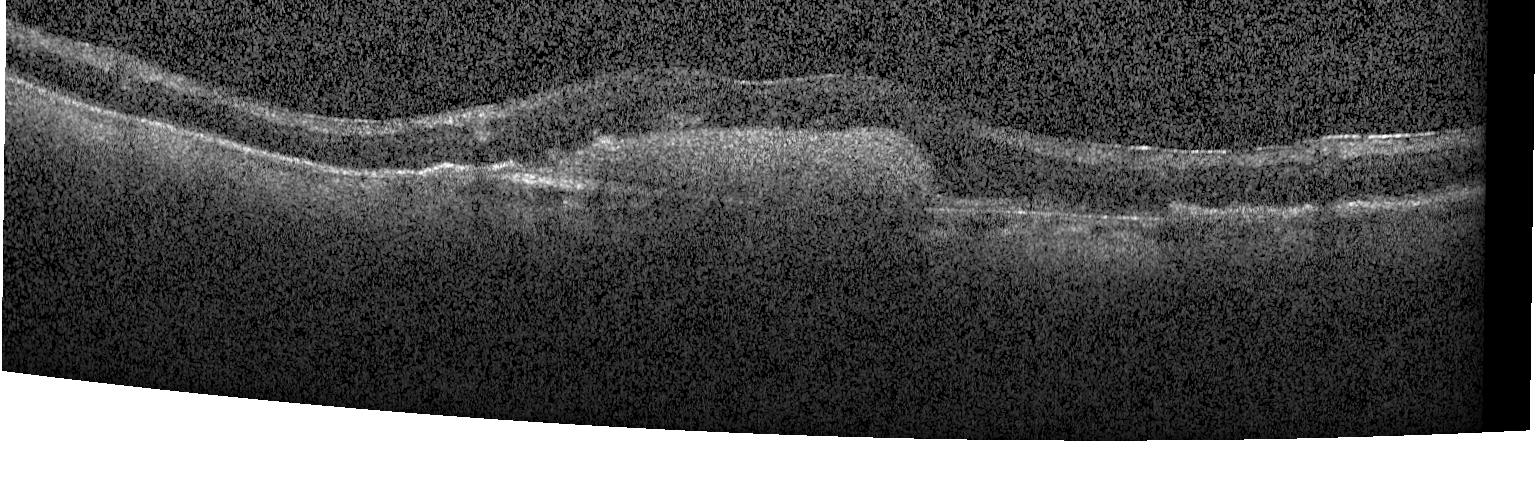 Horizontal scan through the fovea. Instrument: Heidelberg Spectralis. Optical coherence tomography scan — Impression: a choroidal neovascular membrane.